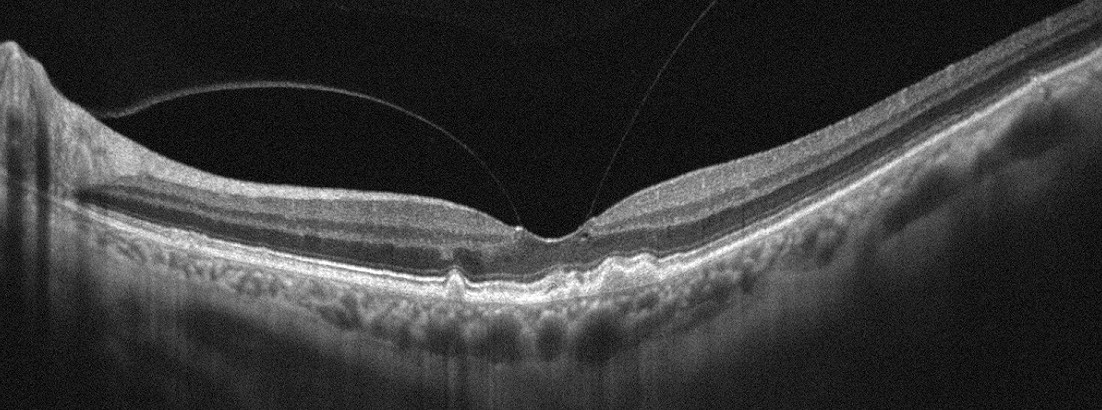
Impression: age-related macular degeneration (AMD).